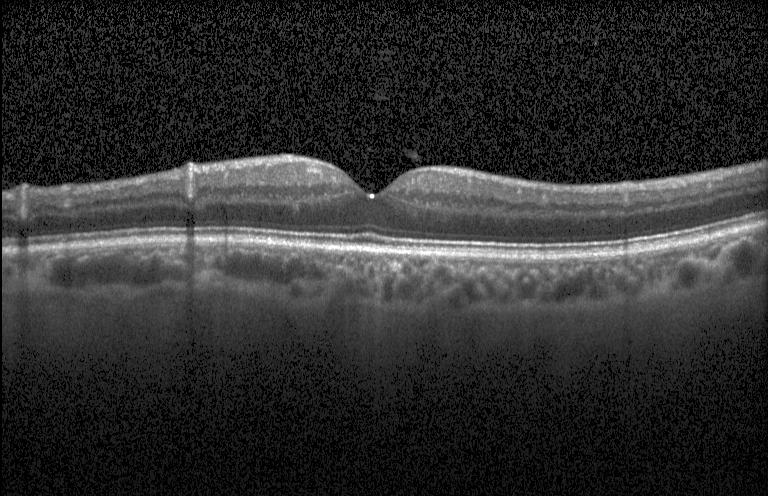
Dx: neither CNV, DME, nor drusen.